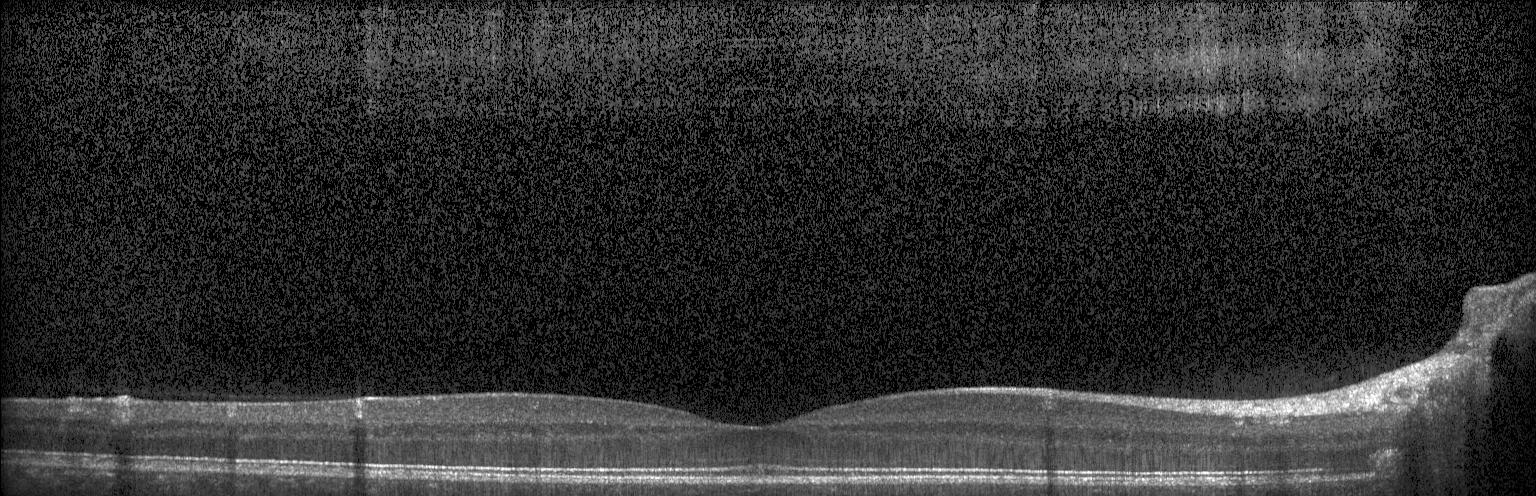 Spectral-domain OCT; OCT B-scan; Heidelberg Spectralis. The scan shows no evidence of choroidal neovascularization, diabetic macular edema, or drusen.